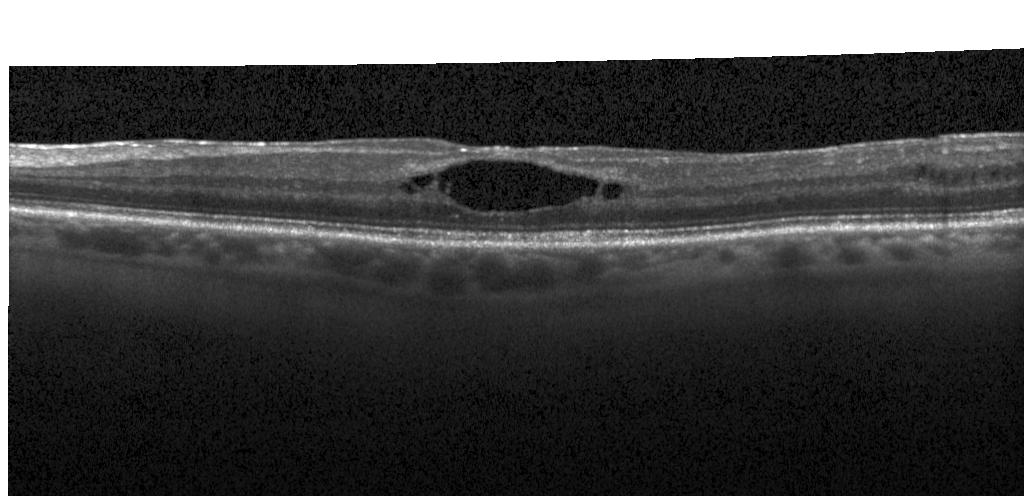
OCT line scan. Finding: diabetic macular edema.